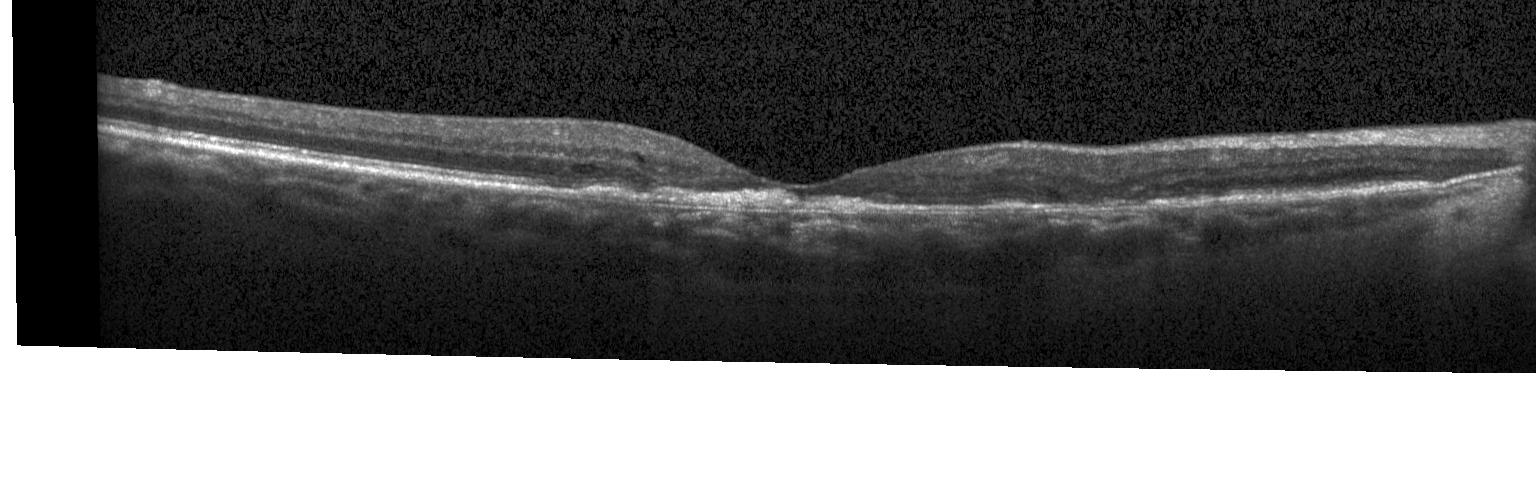
Acquired on a Heidelberg Spectralis. OCT B-scan. Fovea-centered — A choroidal neovascular membrane.